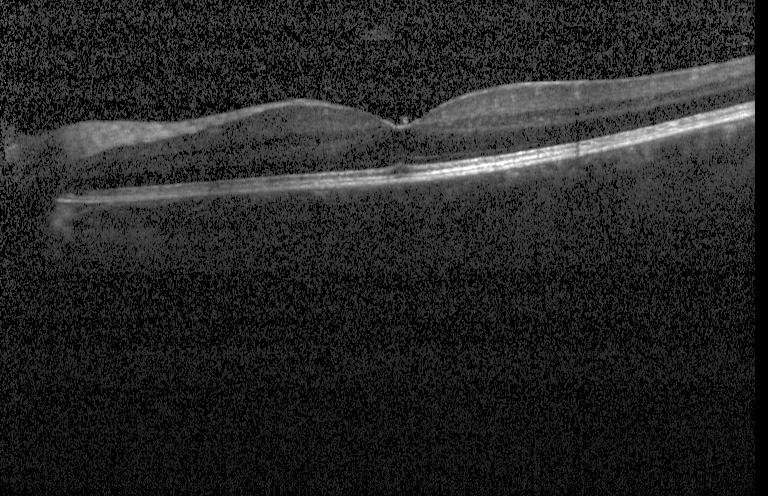 Centered on the fovea, OCT line scan.
No choroidal neovascularization, no diabetic macular edema, and no drusen.